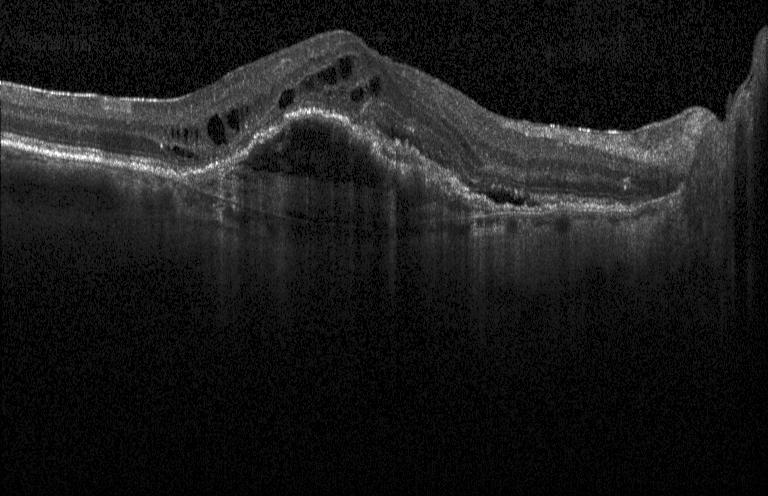
OCT line scan. Macular OCT: choroidal neovascularization.